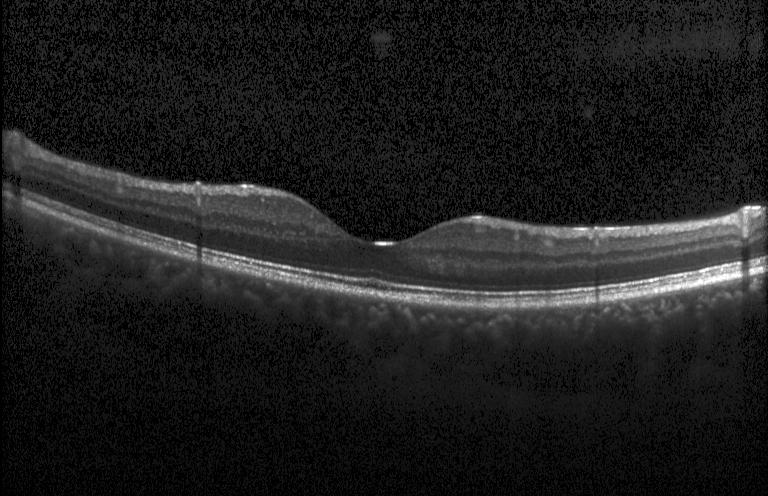

Diagnosis: no choroidal neovascularization, diabetic macular edema, or drusen.